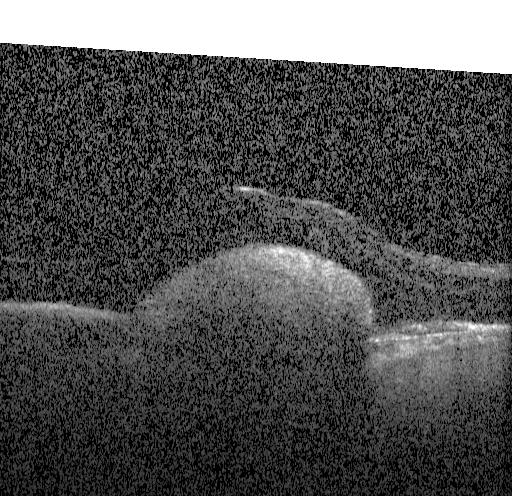
OCT B-scan showing CNV.